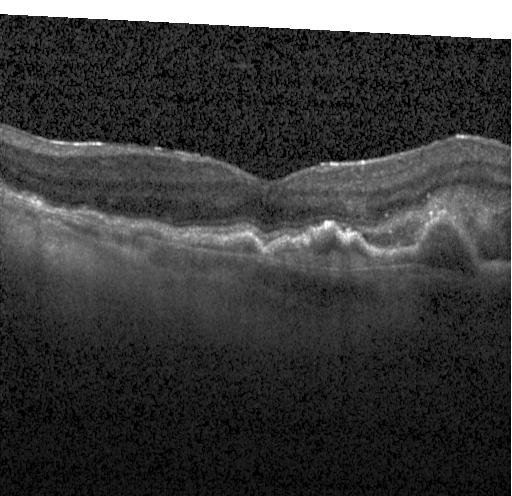
Through the macula. Spectral-domain OCT. Retinal OCT B-scan
Dx: CNV.